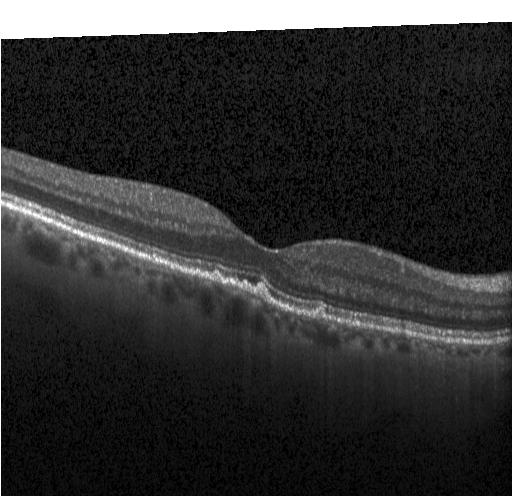

OCT scan showing multiple drusen.